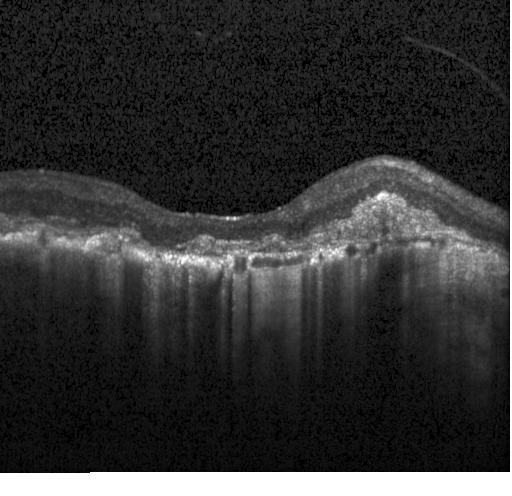 Impression: a choroidal neovascular membrane.